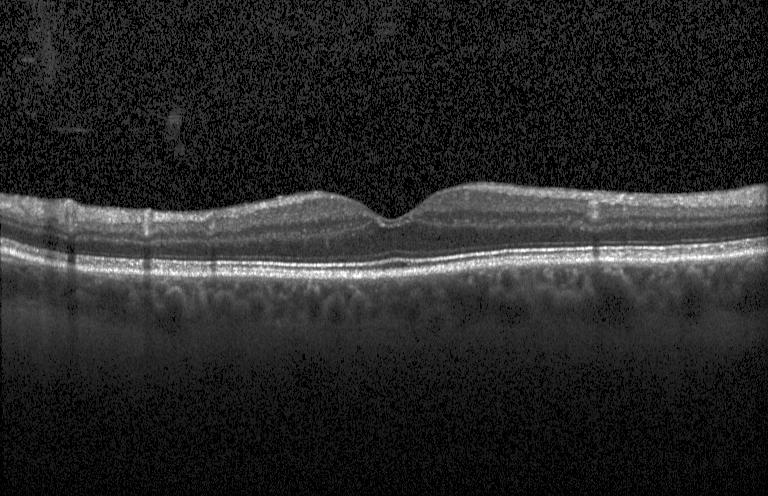 This B-scan demonstrates neither choroidal neovascularization, diabetic macular edema, nor drusen.